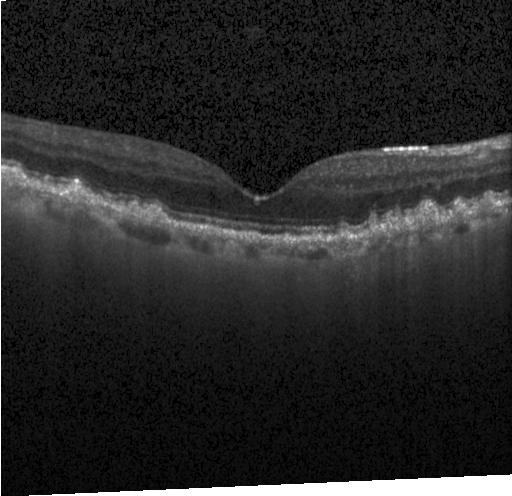 Horizontal scan through the fovea; SD-OCT; optical coherence tomography B-scan — The scan shows multiple drusen.